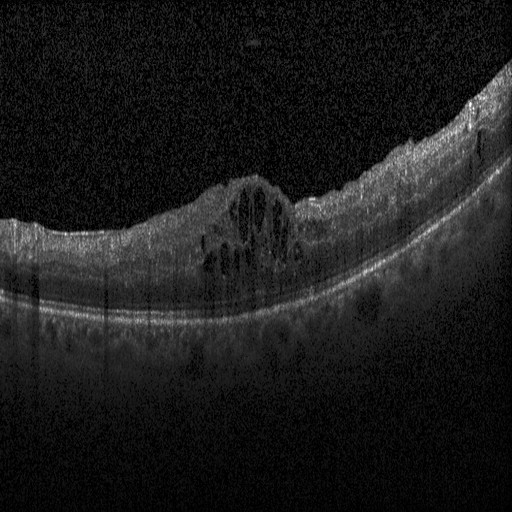
Spectral-domain OCT B-scan: diabetic macular edema.